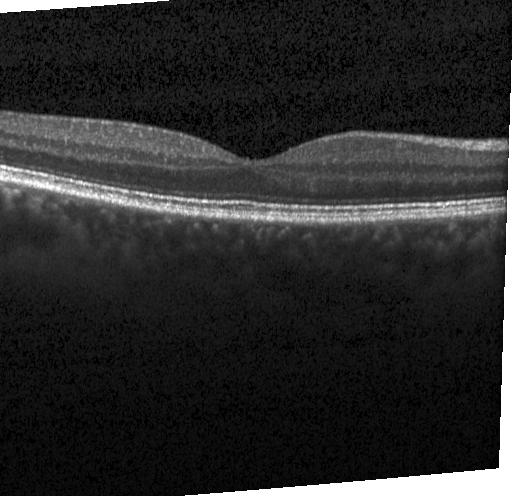

Acquired on a Heidelberg Spectralis, optical coherence tomography B-scan. Finding: no CNV, DME, or drusen.